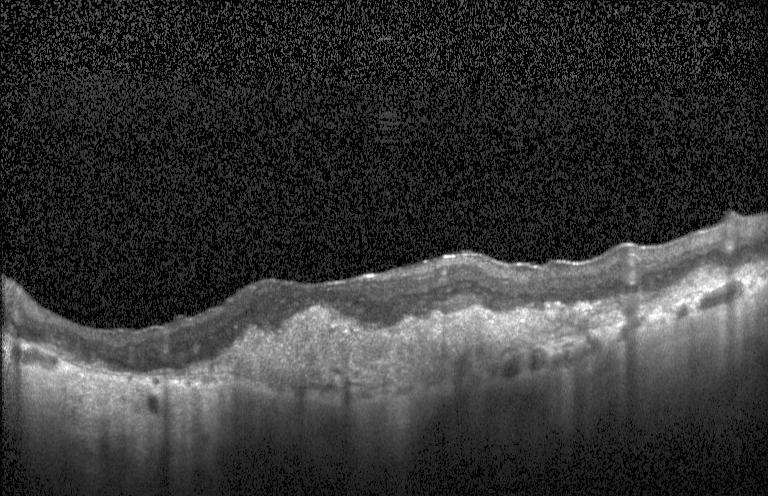 Instrument: Heidelberg Spectralis · OCT B-scan — A choroidal neovascular membrane.